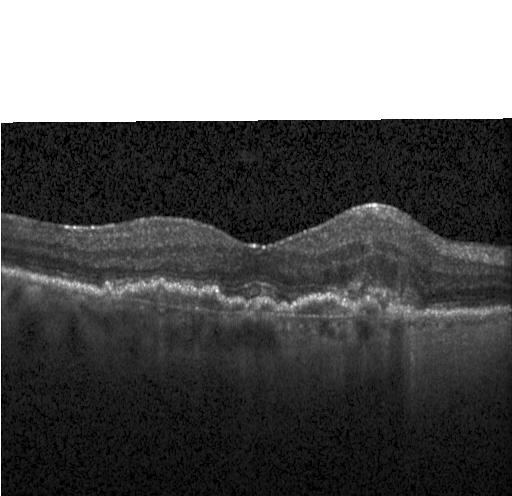 Heidelberg Spectralis, optical coherence tomography scan, spectral-domain OCT.
This B-scan demonstrates choroidal neovascularization.